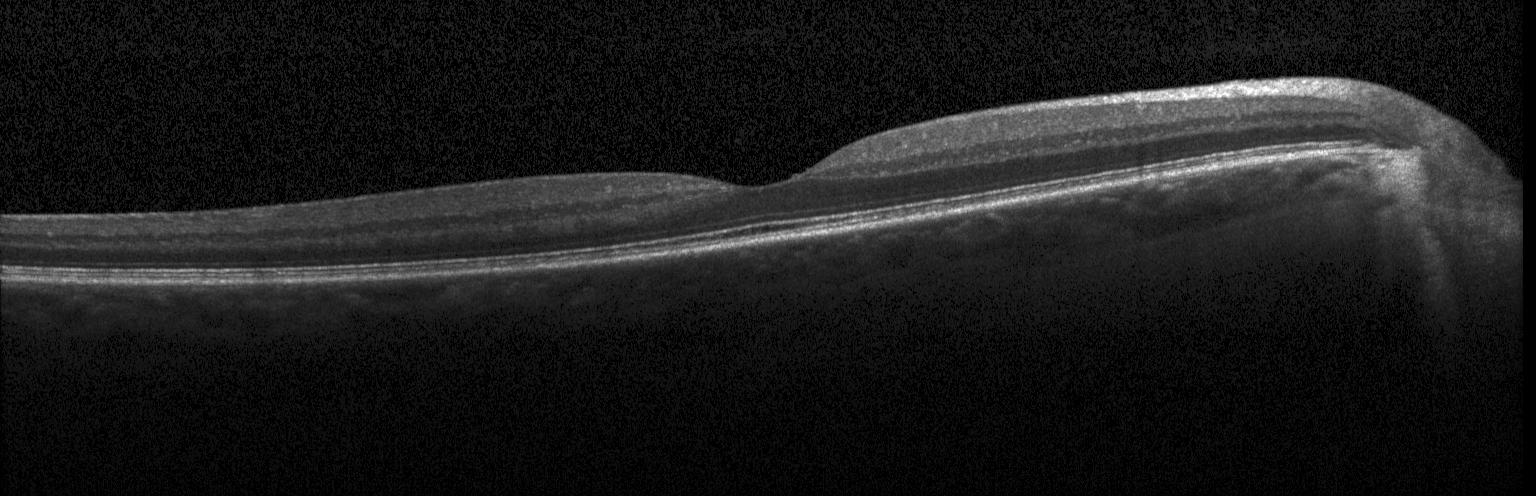 Macular OCT demonstrating neither choroidal neovascularization, diabetic macular edema, nor drusen.